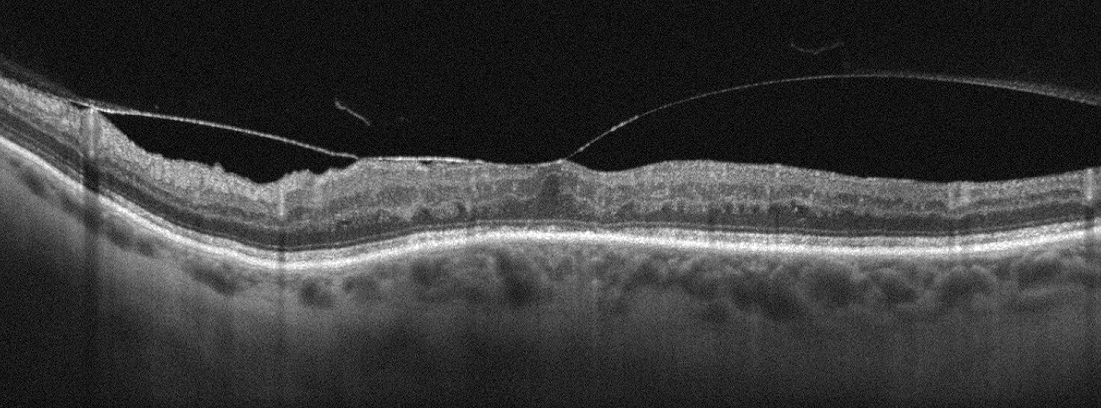 Instrument: Optovue Avanti RTVue XR, optical coherence tomography scan. The scan shows DME.